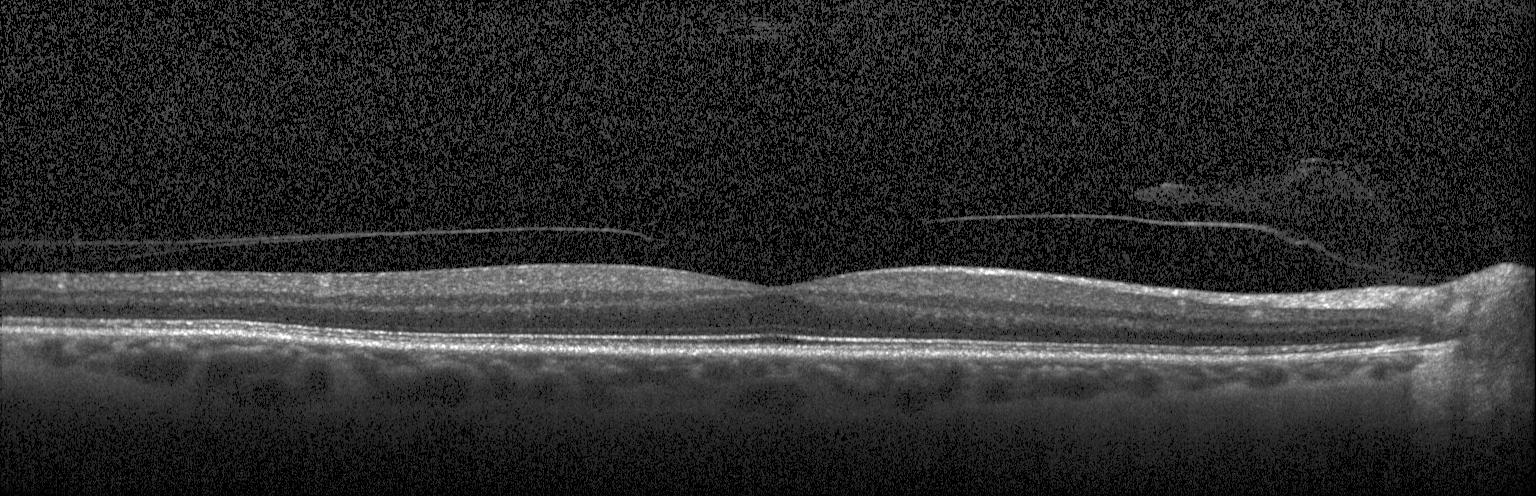 Spectral-domain OCT B-scan: no evidence of choroidal neovascularization, diabetic macular edema, or drusen.